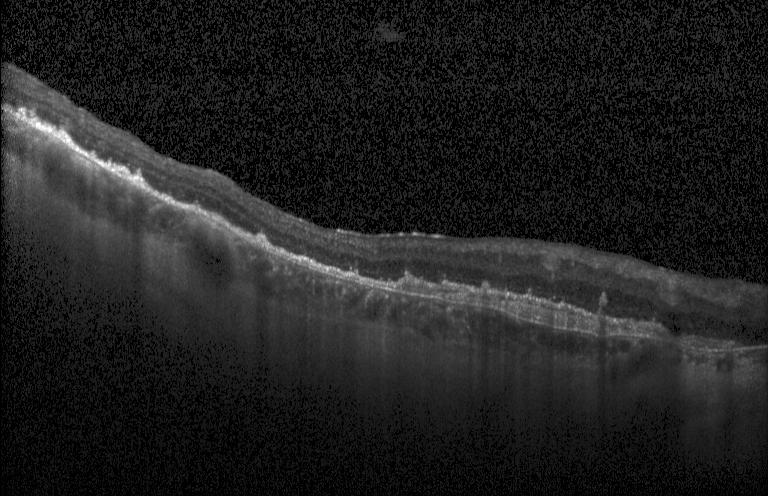 Assessment: a choroidal neovascular membrane.